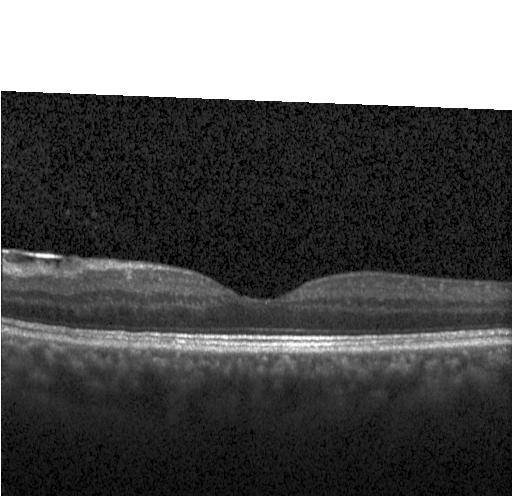
Diagnosis: neither choroidal neovascularization, diabetic macular edema, nor drusen.